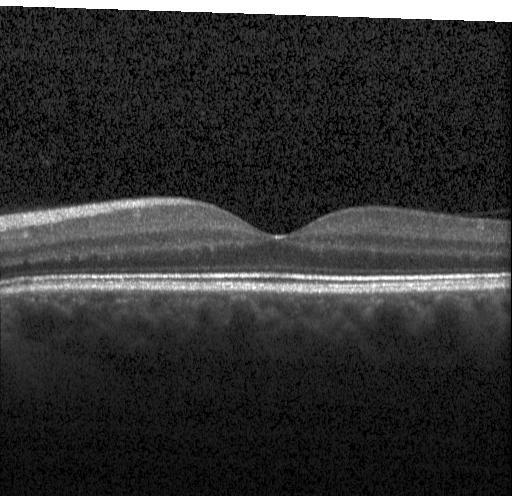

This B-scan demonstrates no choroidal neovascularization, diabetic macular edema, or drusen.